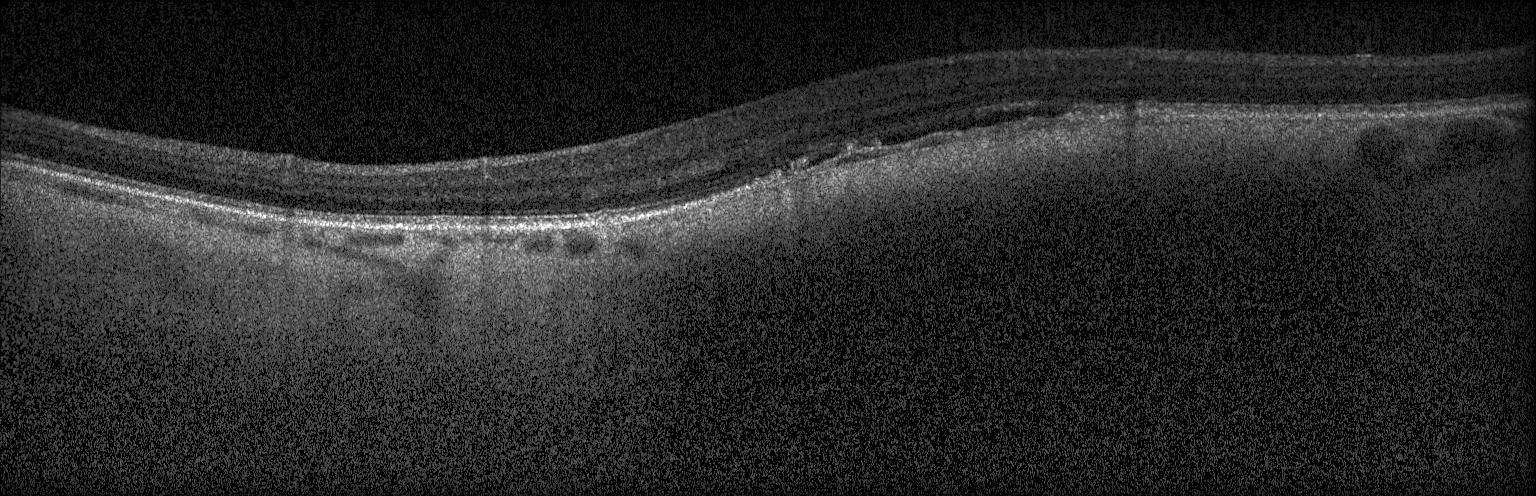
Heidelberg Spectralis OCT system · optical coherence tomography scan · horizontal scan through the fovea — This B-scan demonstrates choroidal neovascularization.